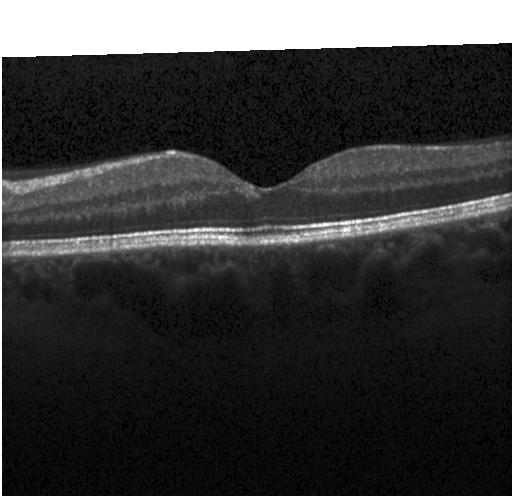
Retinal OCT cross-section; Heidelberg Spectralis OCT system.
The scan shows no choroidal neovascularization, no diabetic macular edema, and no drusen.